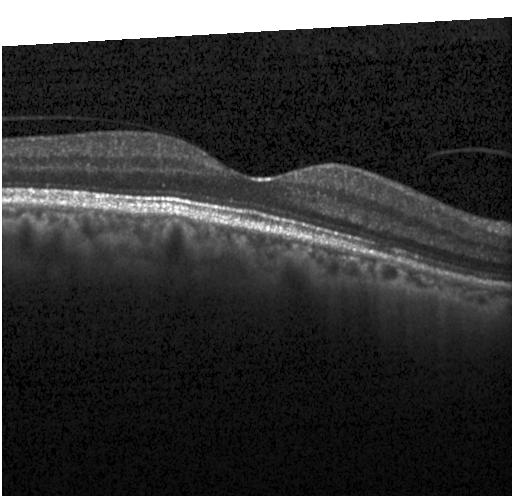
No choroidal neovascularization, no diabetic macular edema, and no drusen.